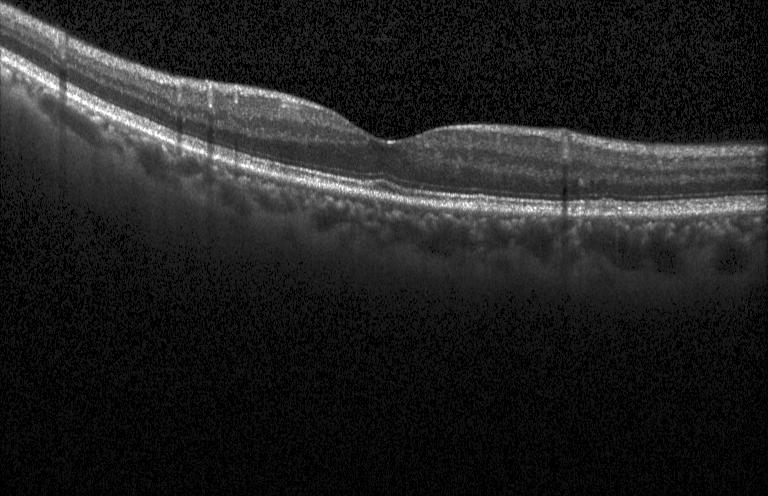
Acquired on a Heidelberg Spectralis · spectral-domain optical coherence tomography · OCT B-scan — Impression: no evidence of choroidal neovascularization, diabetic macular edema, or drusen.